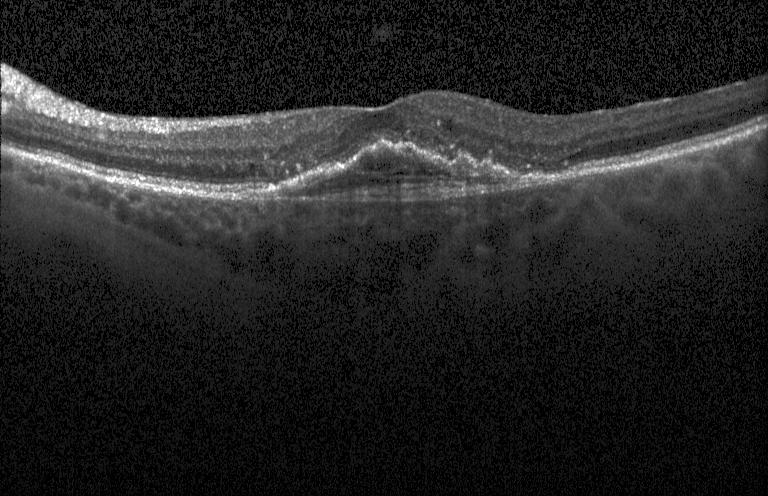 OCT line scan, spectral-domain OCT, fovea-centered
Finding: a choroidal neovascular membrane.